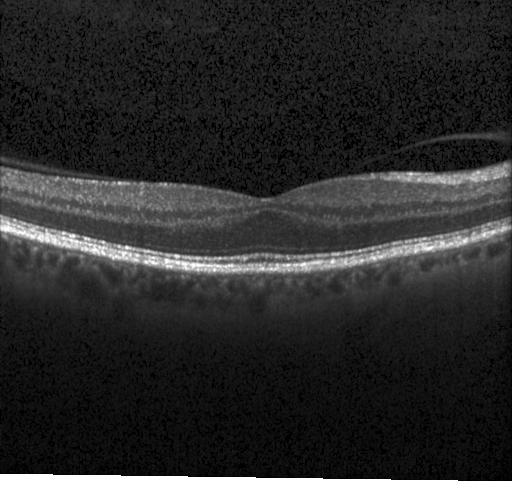 Through the macula · optical coherence tomography scan · acquired on a Heidelberg Spectralis — Diagnosis: neither choroidal neovascularization, diabetic macular edema, nor drusen.